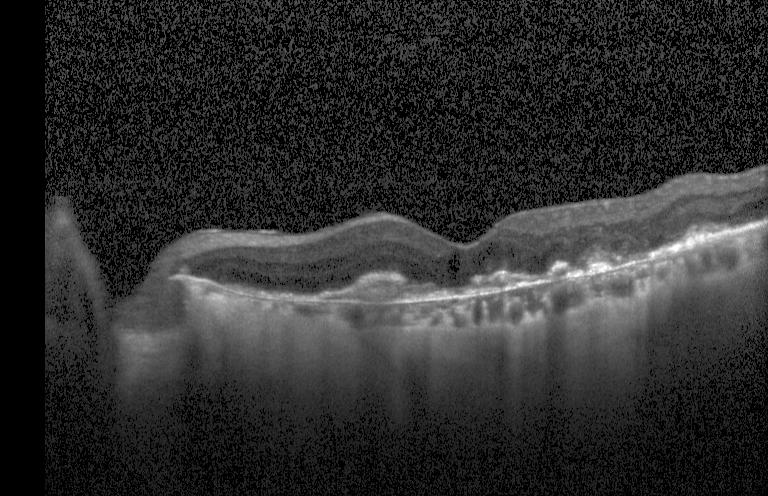
Macular OCT: a choroidal neovascular membrane.